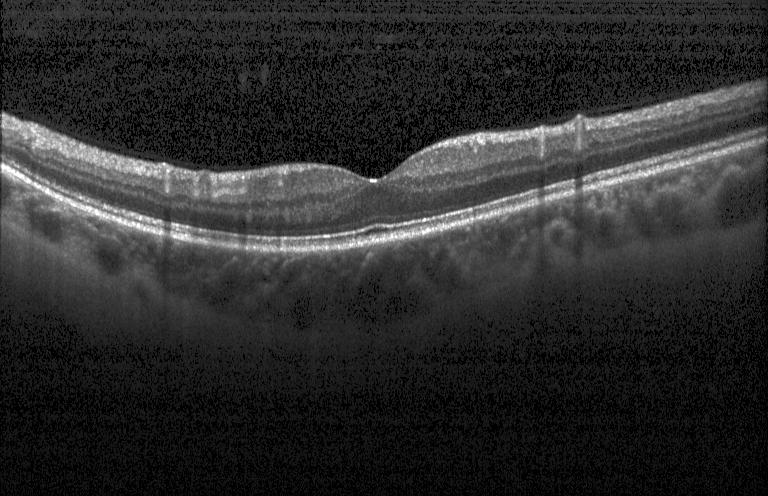 Heidelberg Spectralis; optical coherence tomography B-scan — Diagnosis: no evidence of choroidal neovascularization, diabetic macular edema, or drusen.